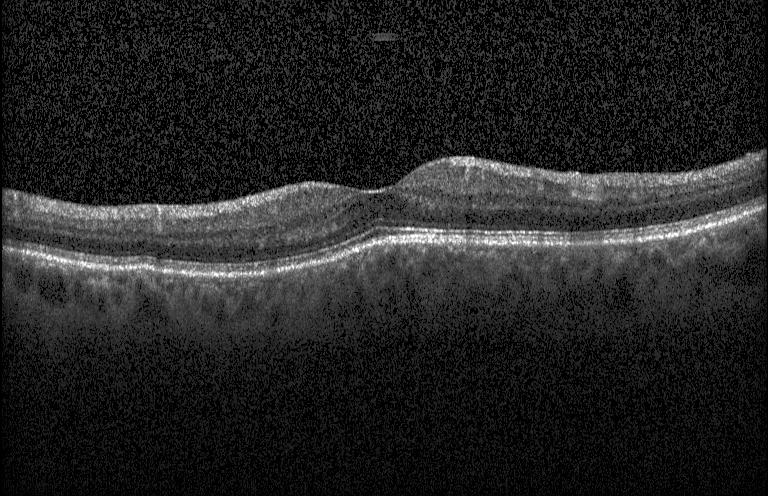

Impression: neither choroidal neovascularization, diabetic macular edema, nor drusen.